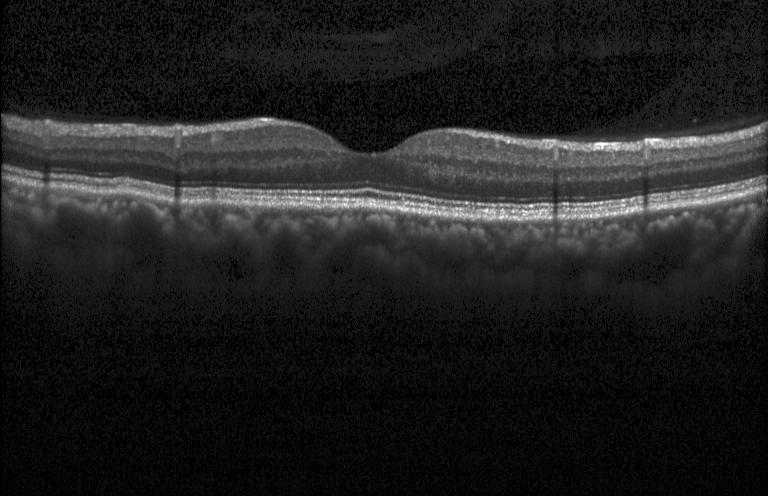
OCT B-scan · acquired on a Heidelberg Spectralis.
Diagnosis: no choroidal neovascularization, diabetic macular edema, or drusen.